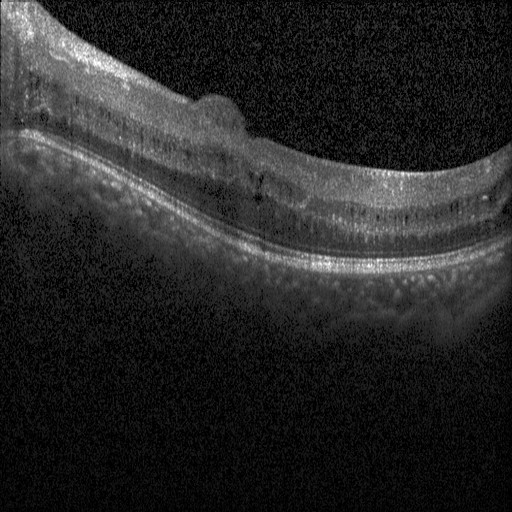
Acquired on a Heidelberg Spectralis · spectral-domain OCT · through the macula · retinal OCT cross-section — The scan shows DME.